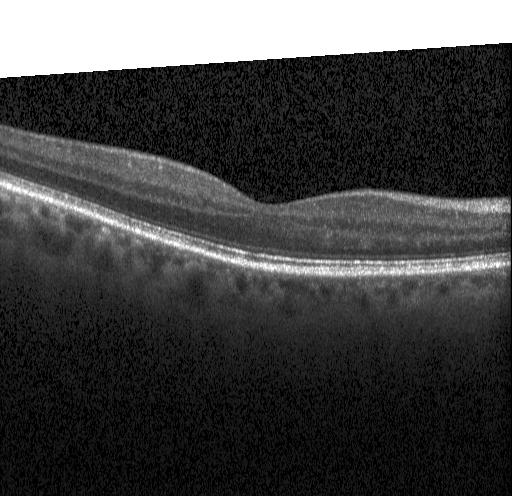
Diagnosis: no evidence of CNV, DME, or drusen.